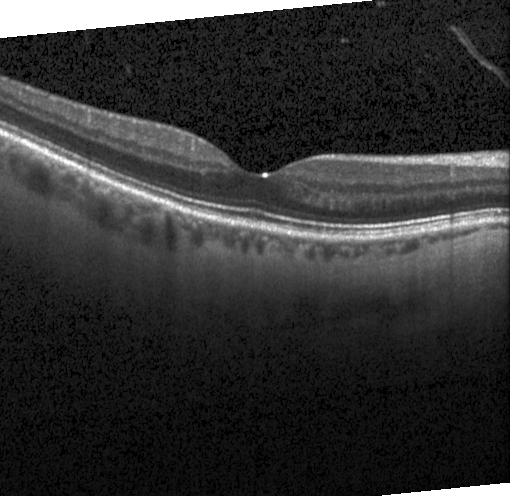

OCT line scan. Dx: no CNV, no DME, and no drusen.